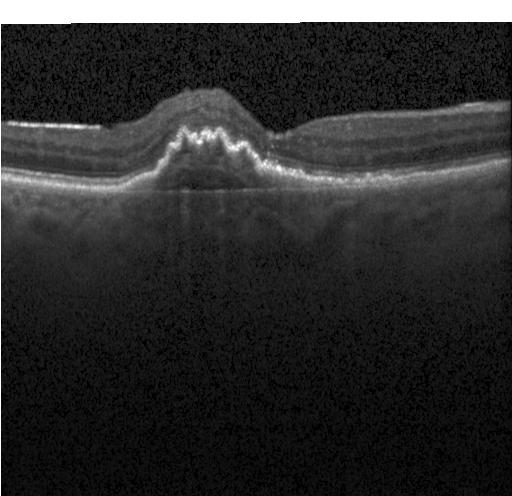
OCT finding: choroidal neovascularization (CNV).